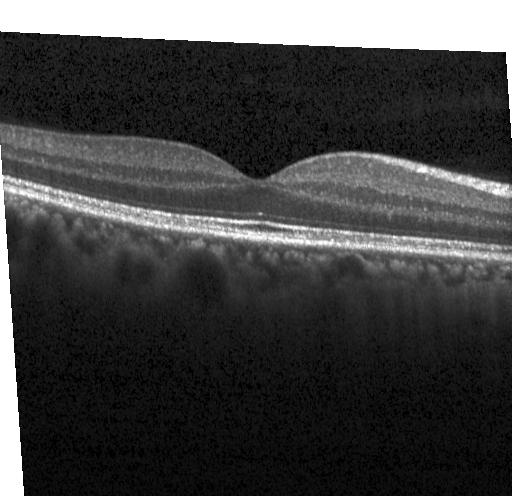
Spectral-domain OCT B-scan: no evidence of CNV, DME, or drusen.